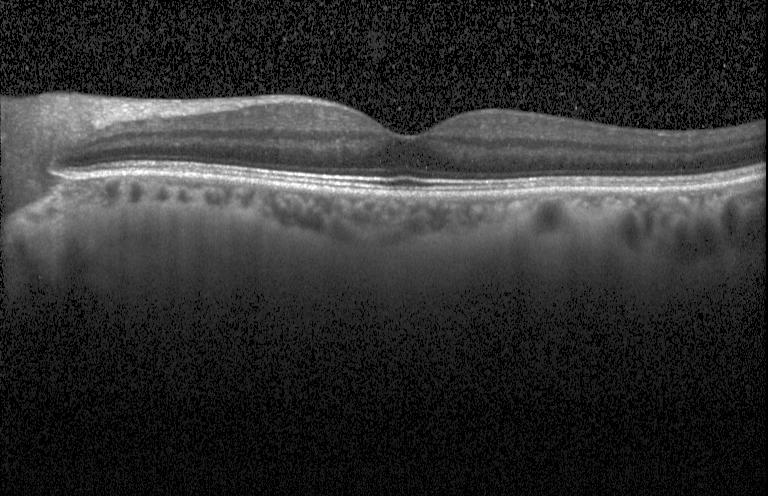 Finding: no CNV, no DME, and no drusen.